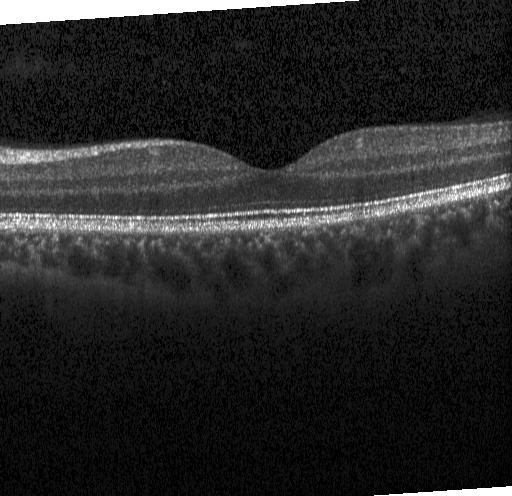 Spectral-domain OCT. OCT B-scan. Horizontal scan through the fovea. Instrument: Heidelberg Spectralis — Diagnosis: no choroidal neovascularization, diabetic macular edema, or drusen.